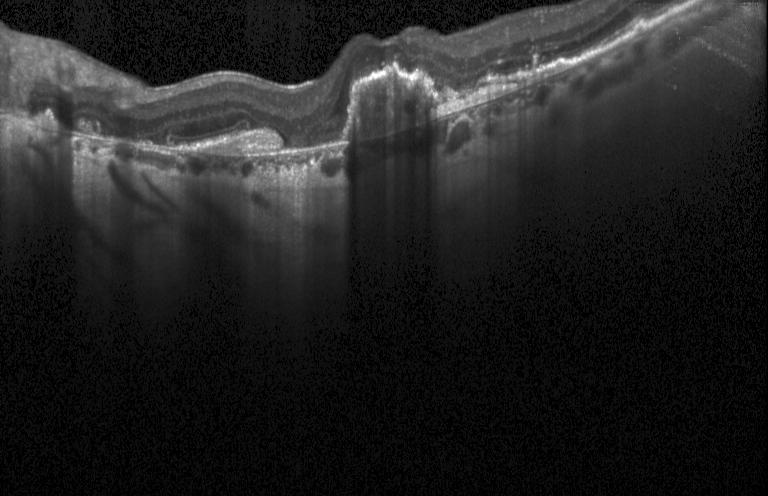
OCT scan showing choroidal neovascularization (CNV).